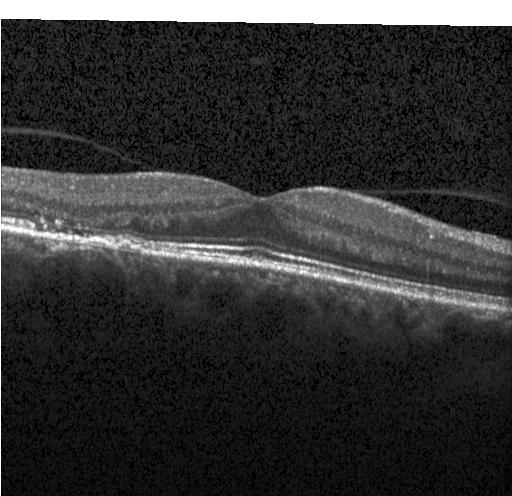

OCT line scan · spectral-domain OCT · instrument: Heidelberg Spectralis — Diagnosis: CNV.